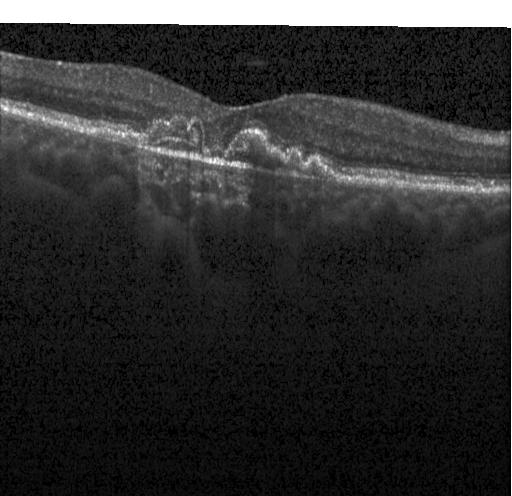

OCT line scan, fovea-centered. The scan shows a choroidal neovascular membrane.